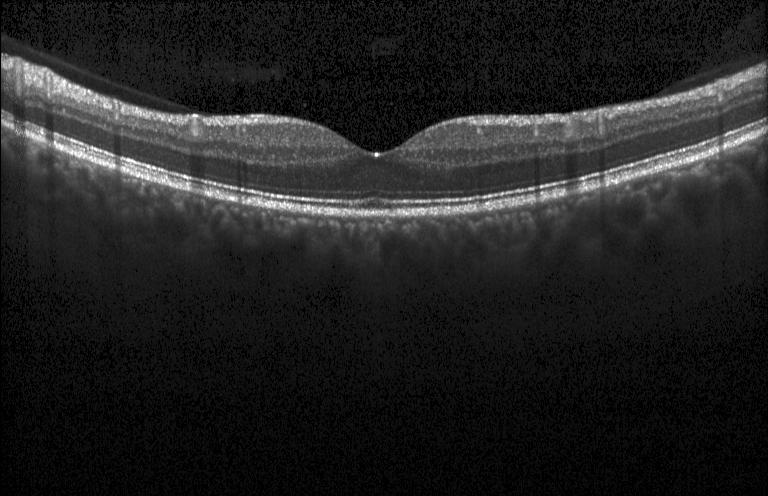

Optical coherence tomography scan
Macular OCT: neither choroidal neovascularization, diabetic macular edema, nor drusen.